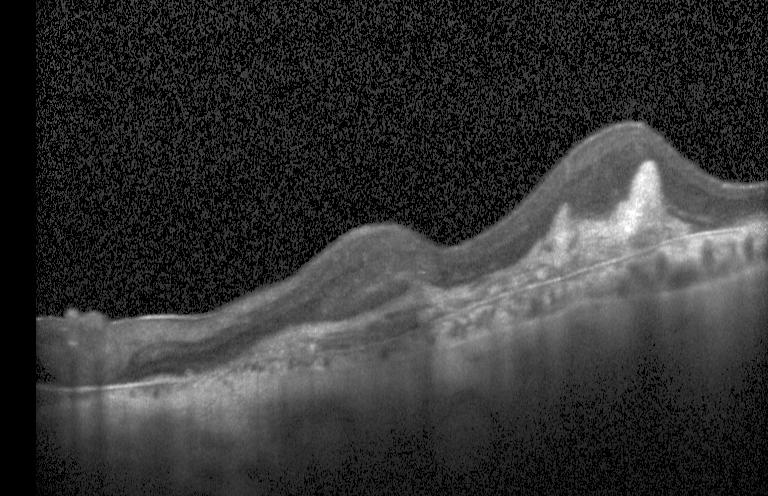 Instrument: Heidelberg Spectralis. Retinal OCT cross-section. SD-OCT. Centered on the fovea — Impression: a choroidal neovascular membrane.